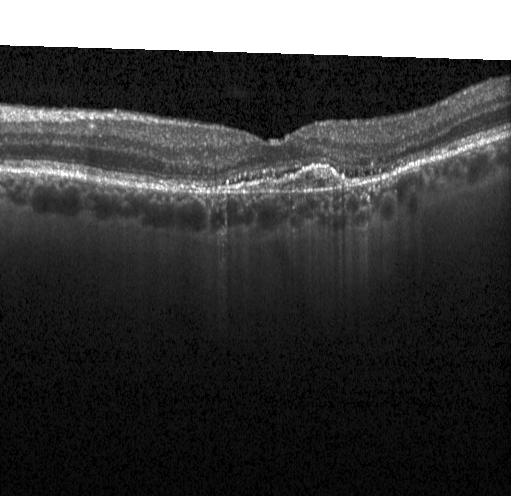
Optical coherence tomography B-scan; centered on the fovea; SD-OCT
Impression: a choroidal neovascular membrane.